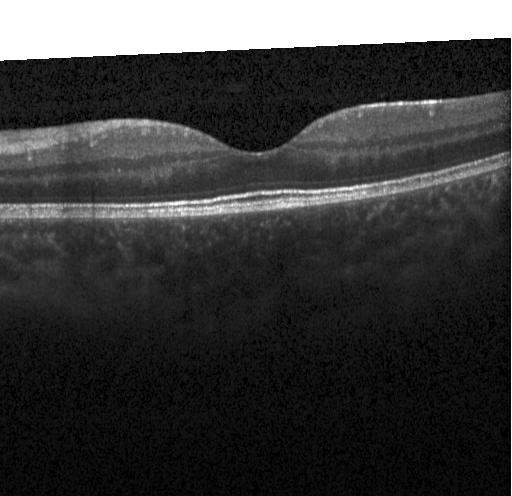

Optical coherence tomography scan.
Diagnosis: no evidence of choroidal neovascularization, diabetic macular edema, or drusen.